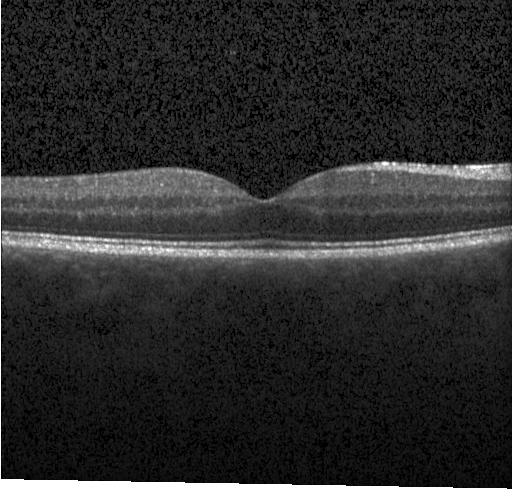
Spectral-domain optical coherence tomography. Optical coherence tomography scan. Fovea-centered.
Finding: no evidence of choroidal neovascularization, diabetic macular edema, or drusen.